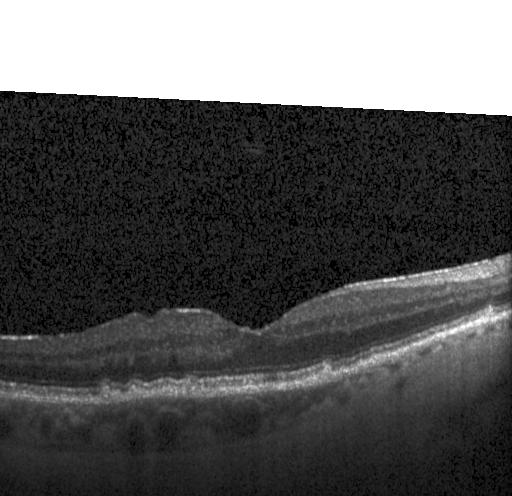

Retinal OCT cross-section, horizontal scan through the fovea.
OCT finding: multiple drusen.